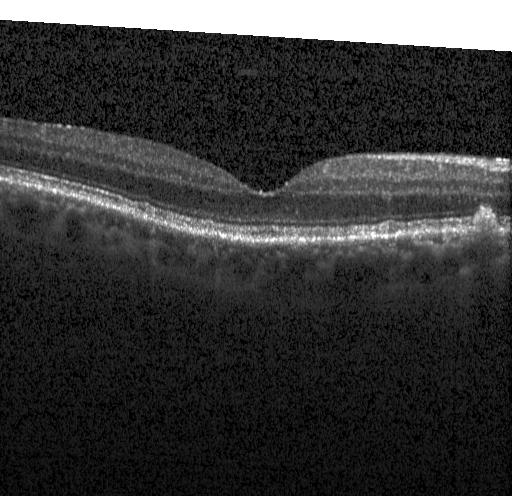 OCT scan showing drusen.